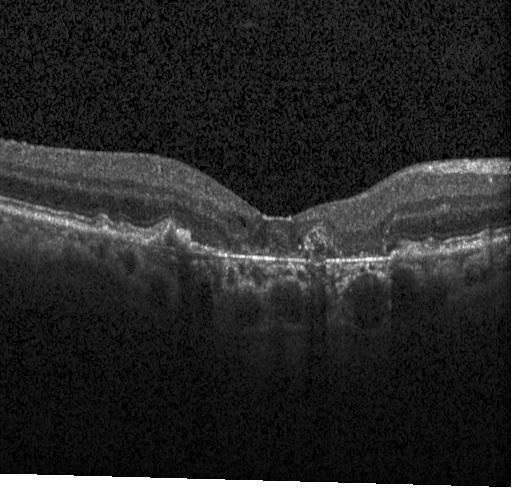

Retinal OCT cross-section. The scan shows a choroidal neovascular membrane.